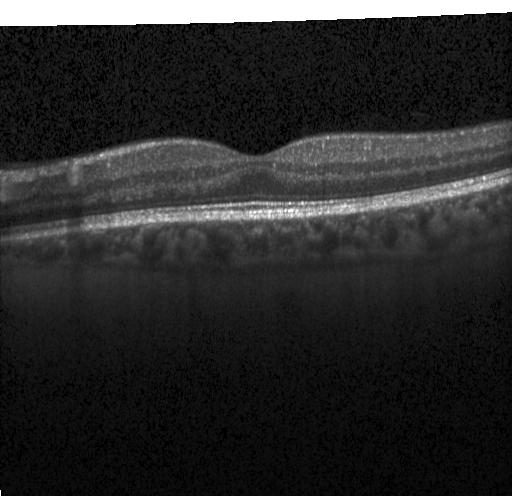 Instrument: Heidelberg Spectralis; OCT B-scan — Impression: neither CNV, DME, nor drusen.